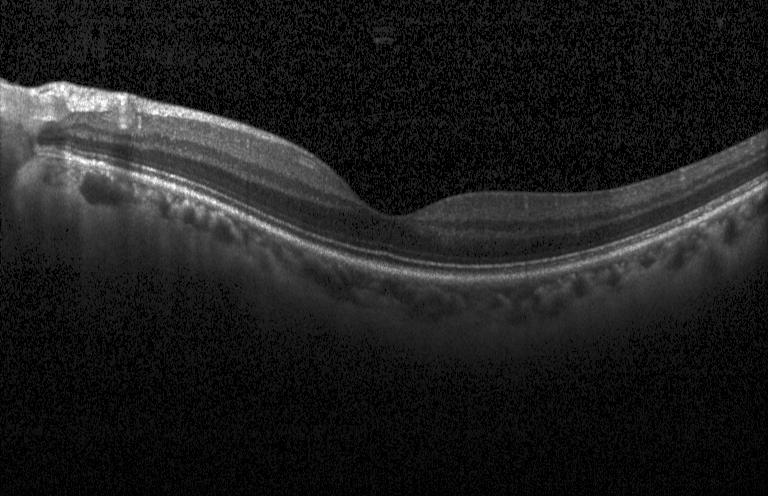

Optical coherence tomography B-scan · spectral-domain optical coherence tomography · instrument: Heidelberg Spectralis.
OCT finding: neither choroidal neovascularization, diabetic macular edema, nor drusen.